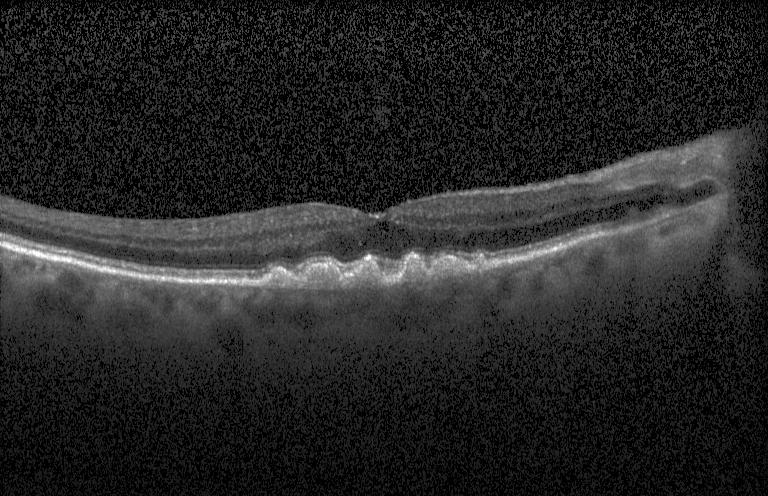
Centered on the fovea, acquired on a Heidelberg Spectralis, optical coherence tomography scan, spectral-domain optical coherence tomography.
Dx: multiple drusen.